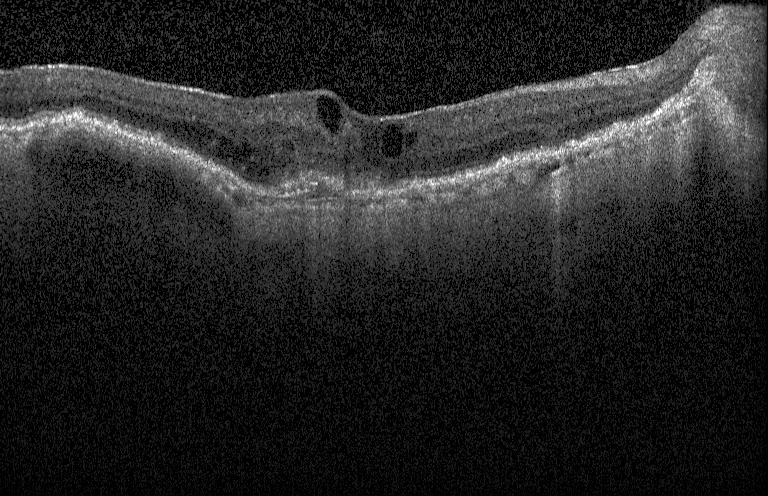
Retinal OCT cross-section showing choroidal neovascularization (CNV).